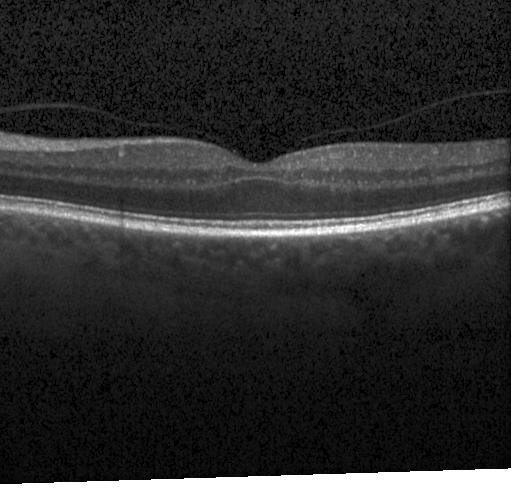
Heidelberg Spectralis OCT system, OCT B-scan — Finding: no choroidal neovascularization, diabetic macular edema, or drusen.